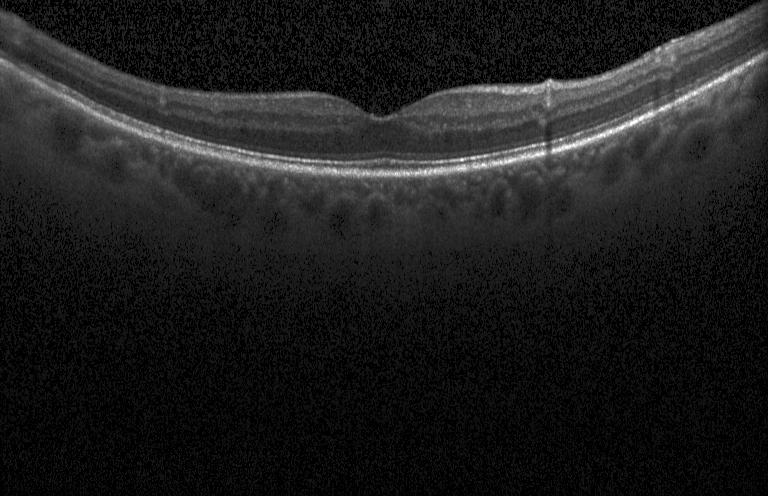

Macular OCT demonstrating neither choroidal neovascularization, diabetic macular edema, nor drusen.